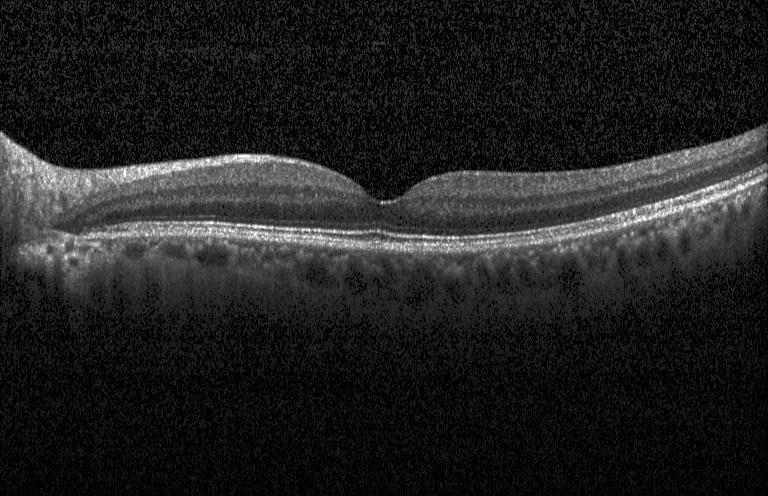

Acquired on a Heidelberg Spectralis. Horizontal scan through the fovea. Optical coherence tomography scan. Spectral-domain optical coherence tomography — No CNV, no DME, and no drusen.